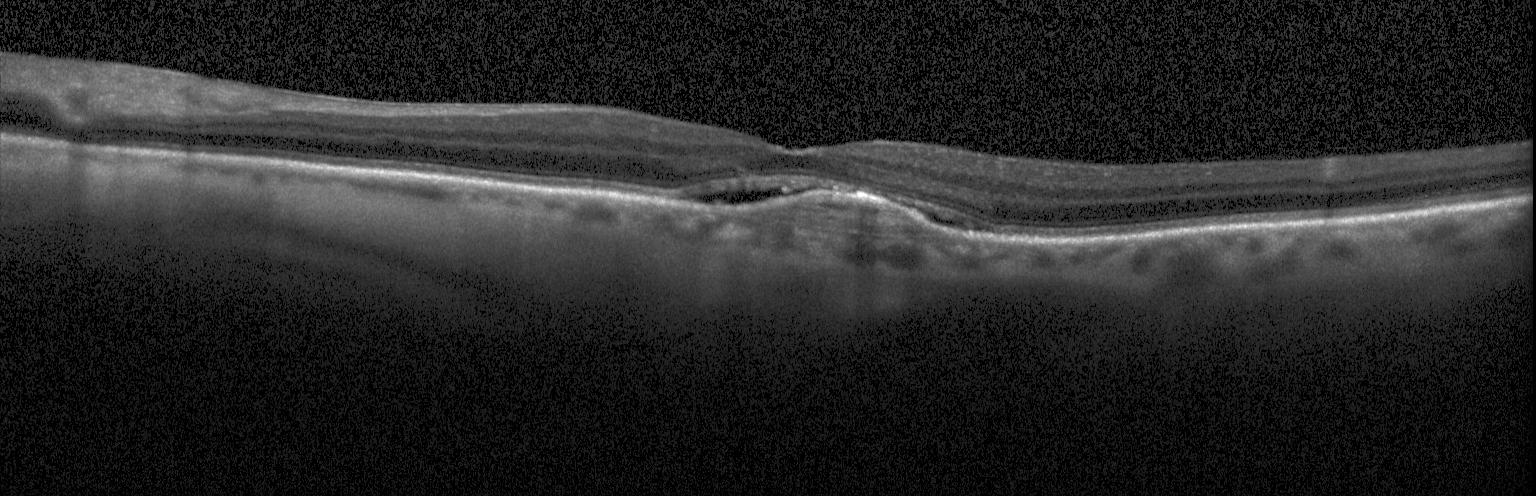 Fovea-centered. Retinal OCT B-scan
Impression: choroidal neovascularization (CNV).